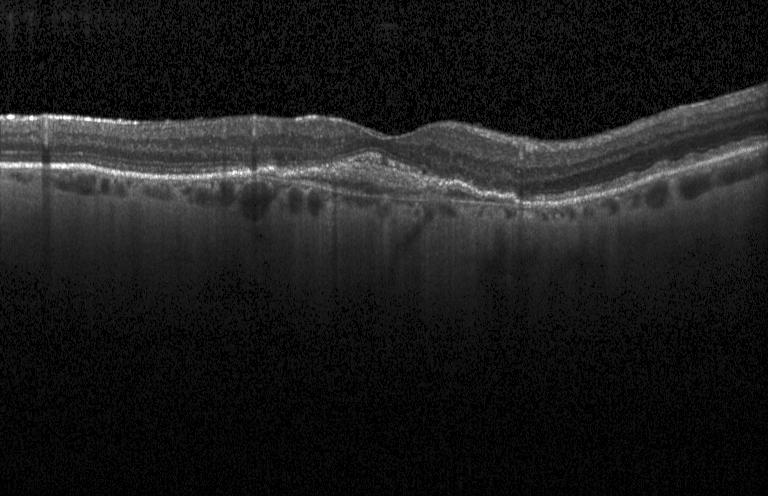

Spectral-domain OCT B-scan: a choroidal neovascular membrane.